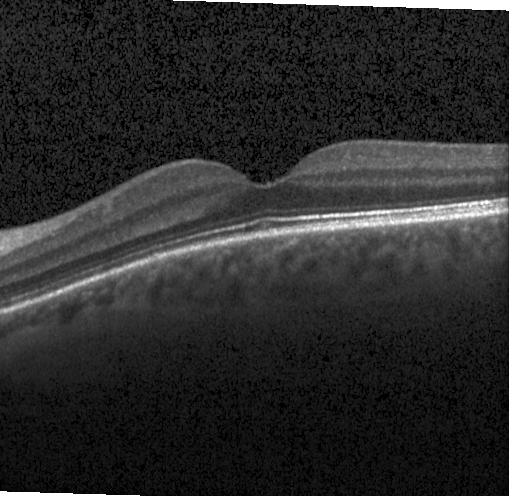 Spectral-domain OCT B-scan: no evidence of CNV, DME, or drusen.